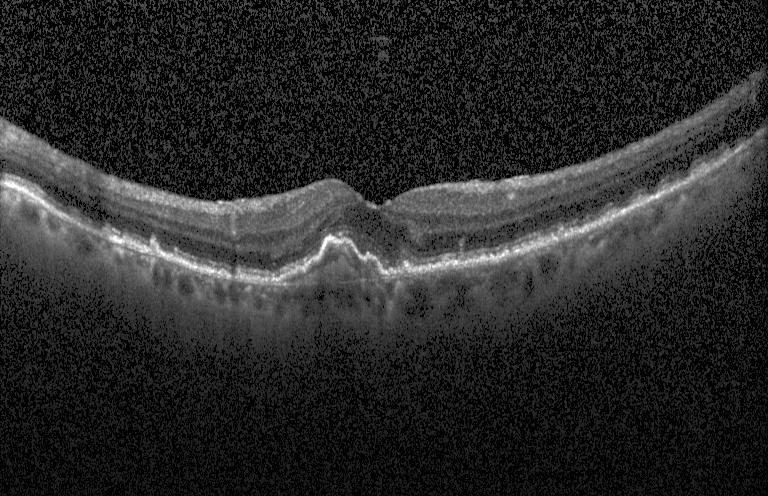
Retinal OCT cross-section, SD-OCT.
Impression: choroidal neovascularization (CNV).